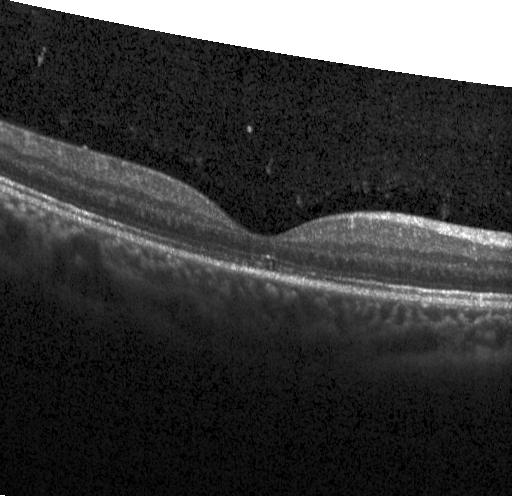

Optical coherence tomography B-scan · Heidelberg Spectralis · spectral-domain OCT — The scan shows no choroidal neovascularization, diabetic macular edema, or drusen.